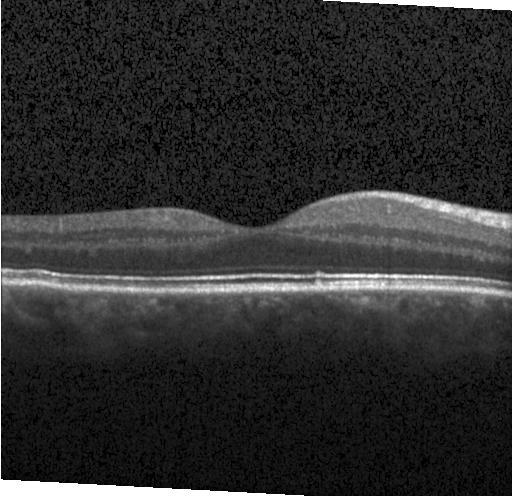

OCT B-scan showing multiple drusen.